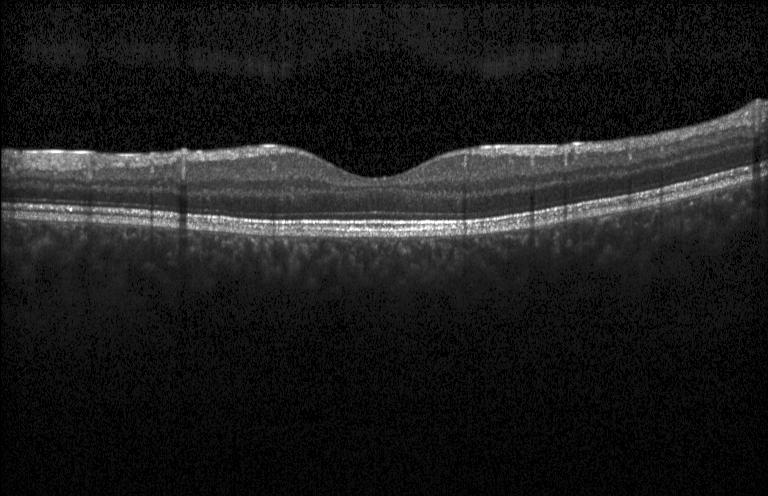
Diagnosis: no choroidal neovascularization, no diabetic macular edema, and no drusen.